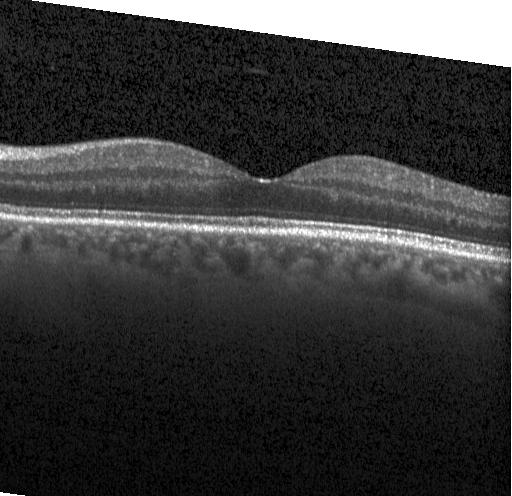 Acquired on a Heidelberg Spectralis, centered on the fovea, OCT B-scan, SD-OCT
Diagnosis: no choroidal neovascularization, no diabetic macular edema, and no drusen.